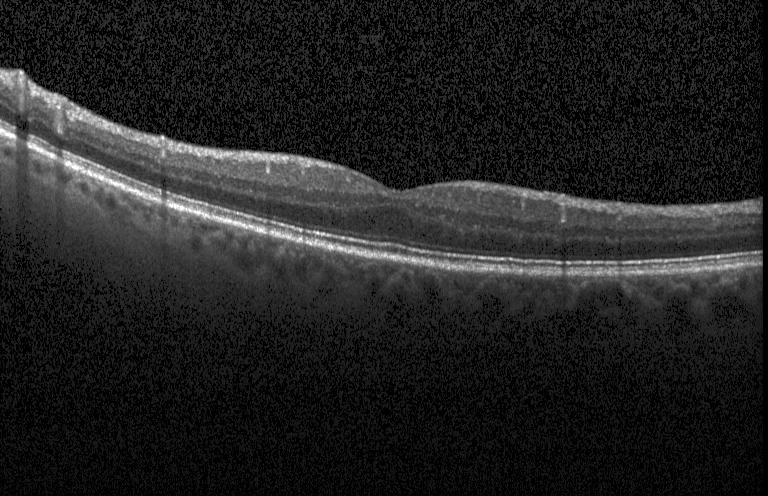

Spectral-domain optical coherence tomography, horizontal scan through the fovea, retinal OCT cross-section — Finding: no choroidal neovascularization, no diabetic macular edema, and no drusen.